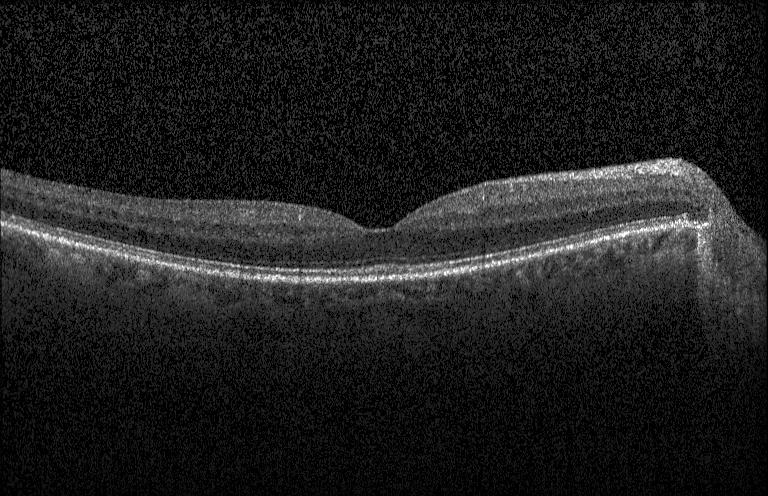 Retinal OCT B-scan.
Assessment: no CNV, no DME, and no drusen.